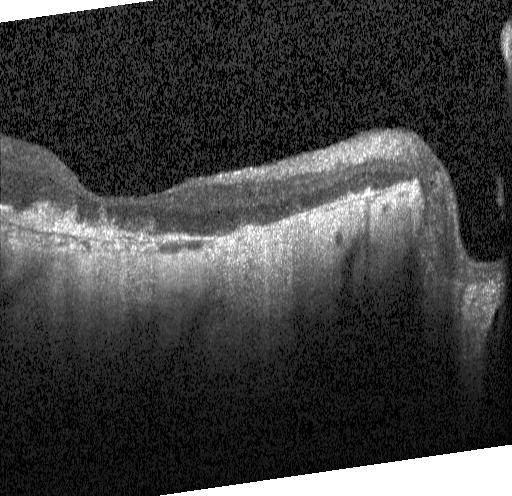 Retinal OCT cross-section — This B-scan demonstrates choroidal neovascularization.